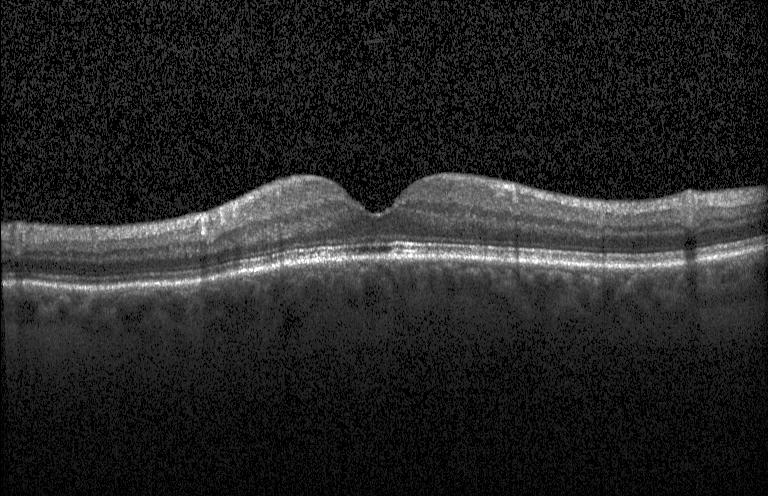 Finding: no choroidal neovascularization, no diabetic macular edema, and no drusen.